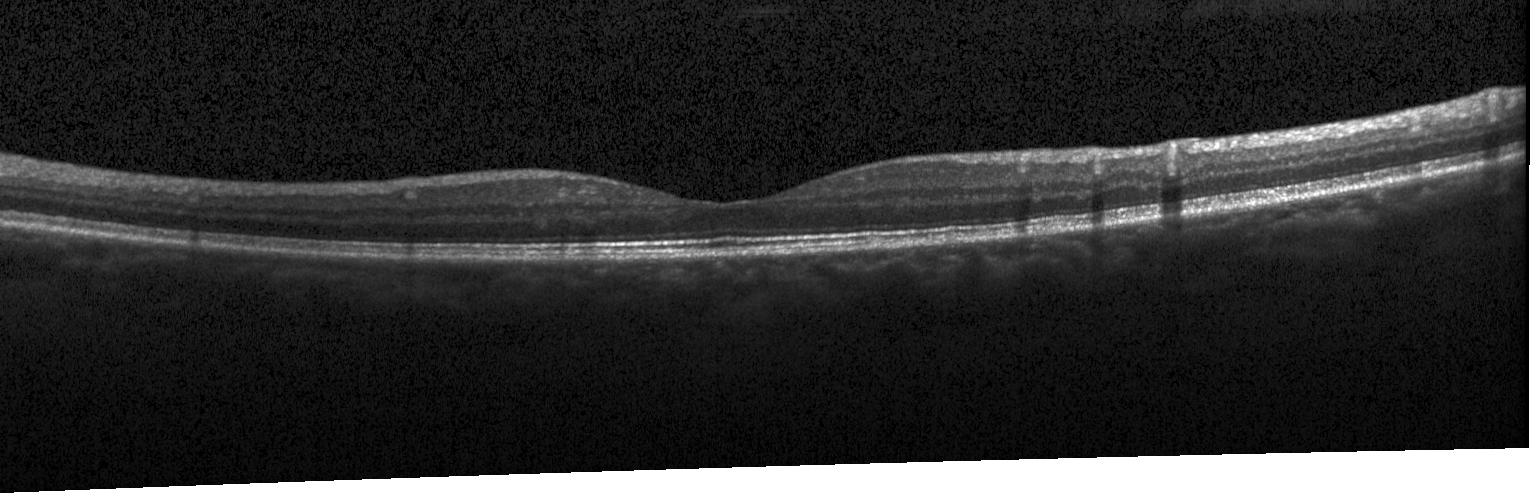

Fovea-centered, retinal OCT cross-section. Impression: neither choroidal neovascularization, diabetic macular edema, nor drusen.